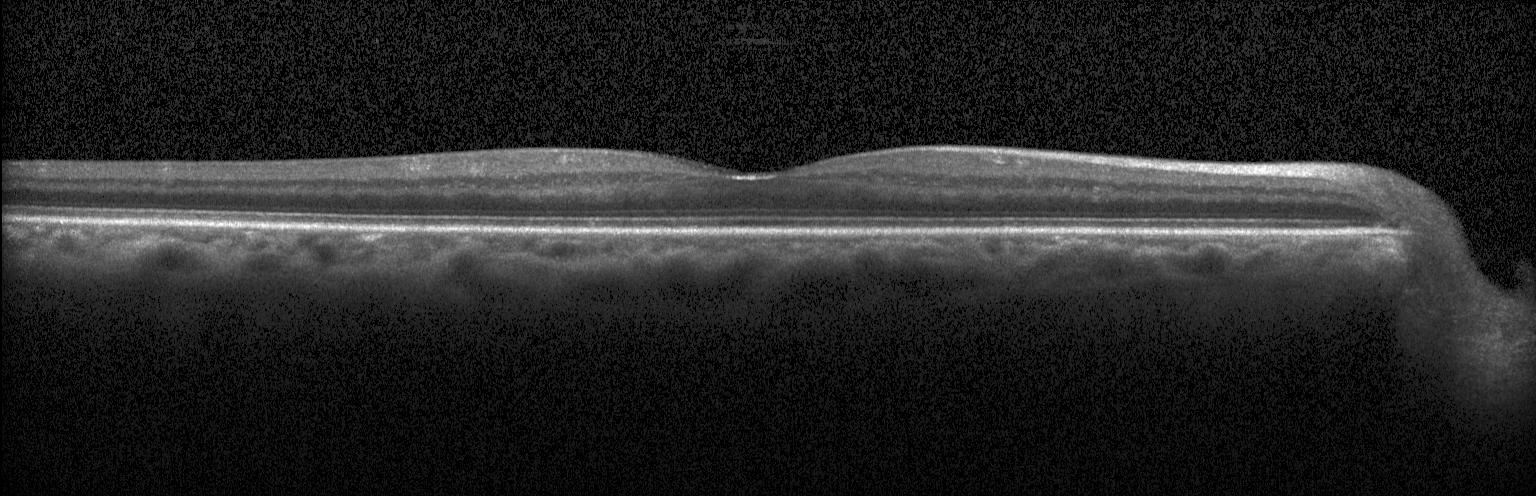

Horizontal scan through the fovea. Optical coherence tomography scan. Instrument: Heidelberg Spectralis — Diagnosis: no CNV, no DME, and no drusen.